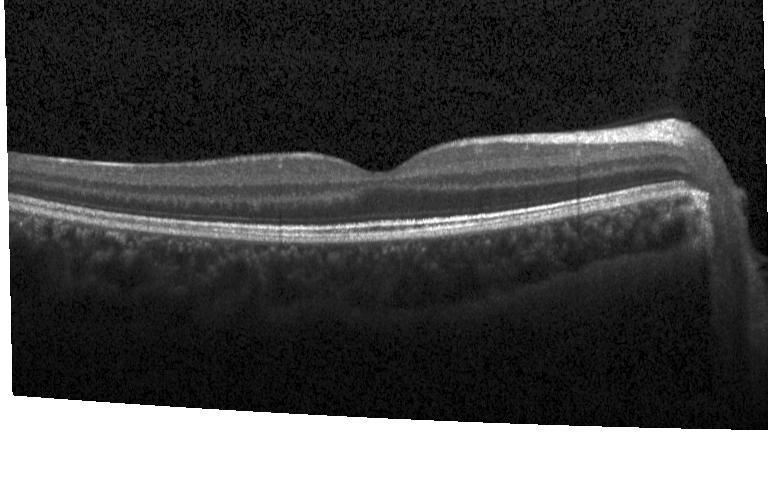 OCT line scan. Heidelberg Spectralis OCT system — Macular OCT: no choroidal neovascularization, diabetic macular edema, or drusen.